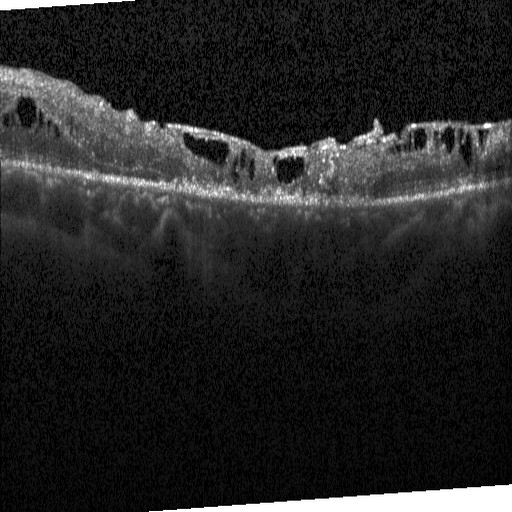

Impression: DME.